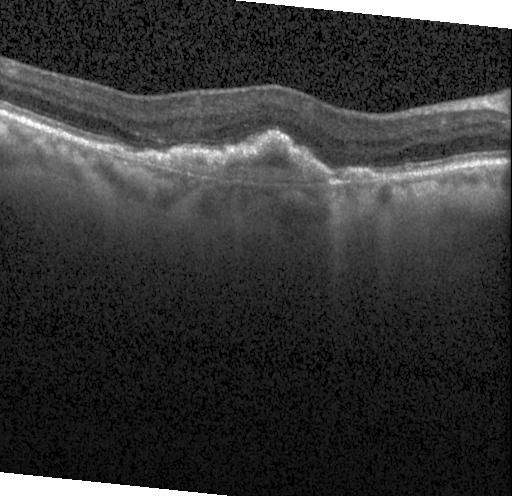
Heidelberg Spectralis OCT system. Spectral-domain OCT. Optical coherence tomography B-scan. Horizontal scan through the fovea — Assessment: a choroidal neovascular membrane.